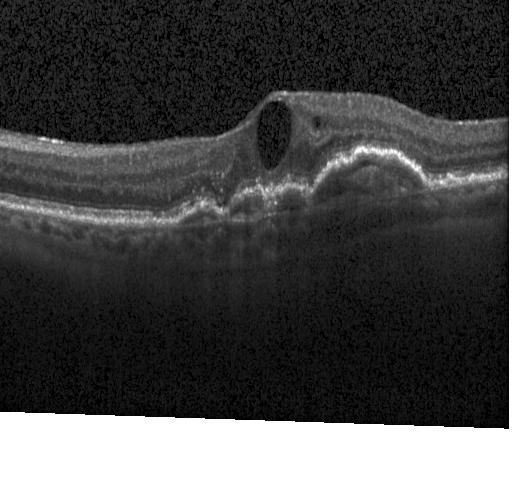
Centered on the fovea, optical coherence tomography scan. Diagnosis: CNV.